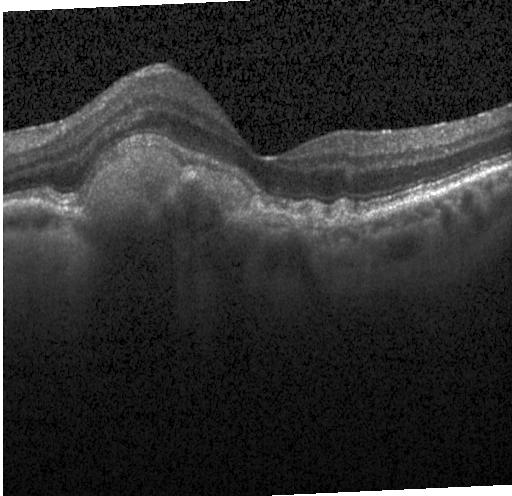

Macular scan · spectral-domain optical coherence tomography · retinal OCT cross-section · Heidelberg Spectralis — Diagnosis: a choroidal neovascular membrane.